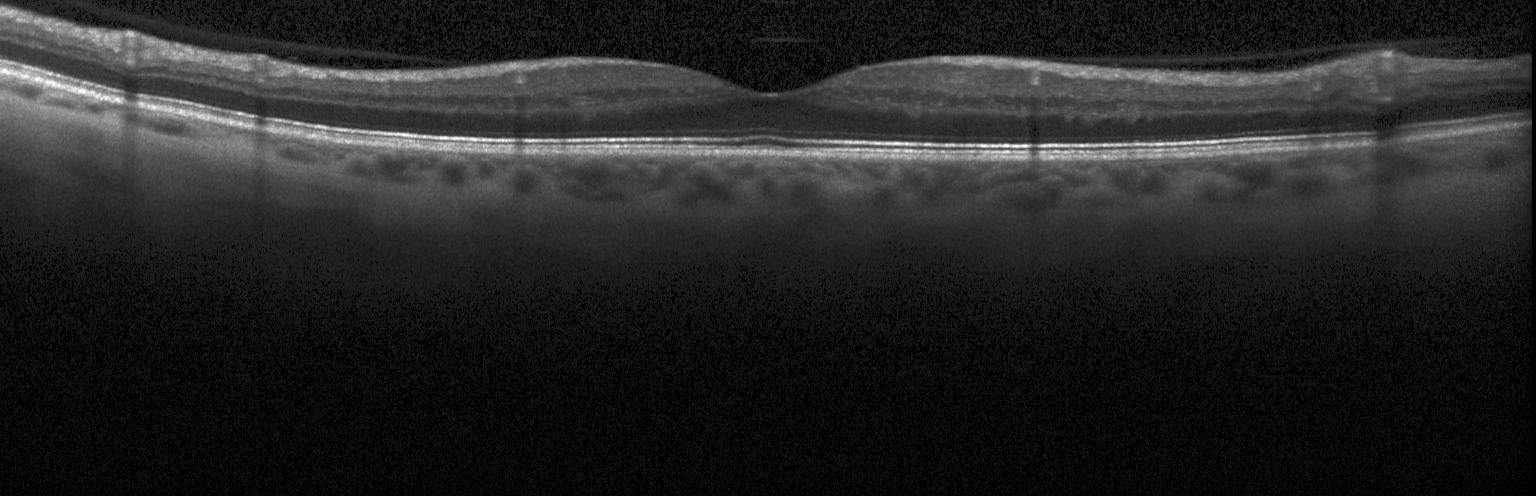
No choroidal neovascularization, diabetic macular edema, or drusen.